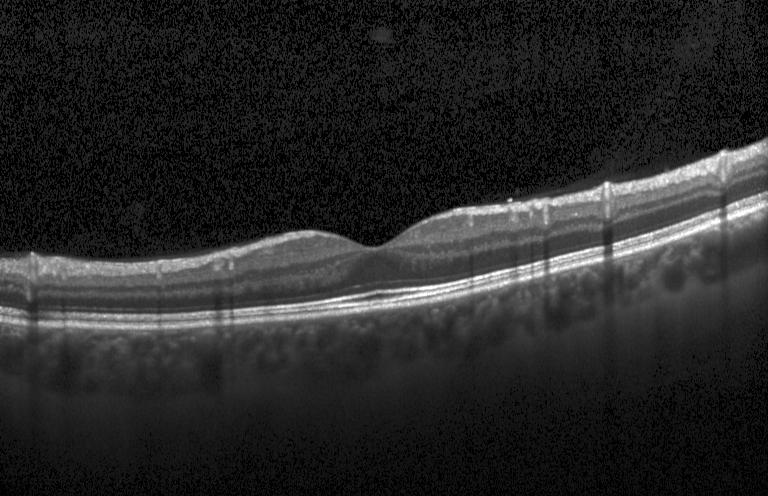

OCT scan showing no choroidal neovascularization, diabetic macular edema, or drusen.